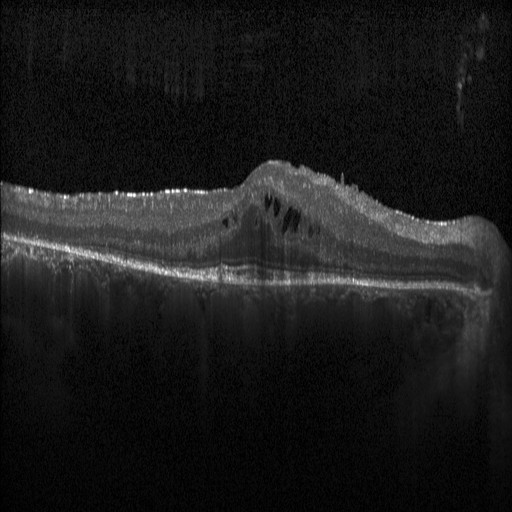

Horizontal scan through the fovea; spectral-domain optical coherence tomography; OCT B-scan.
Macular OCT: diabetic macular edema.